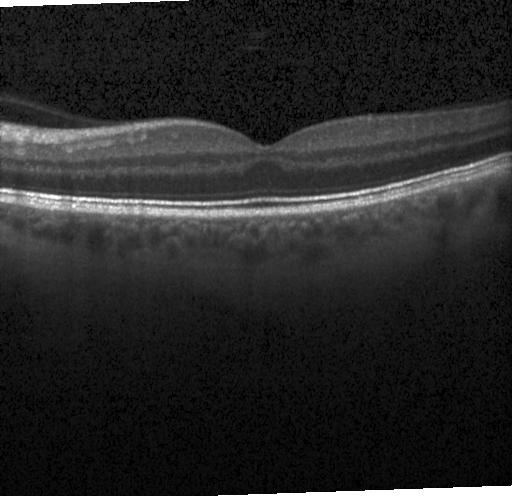

Macular OCT: neither CNV, DME, nor drusen.